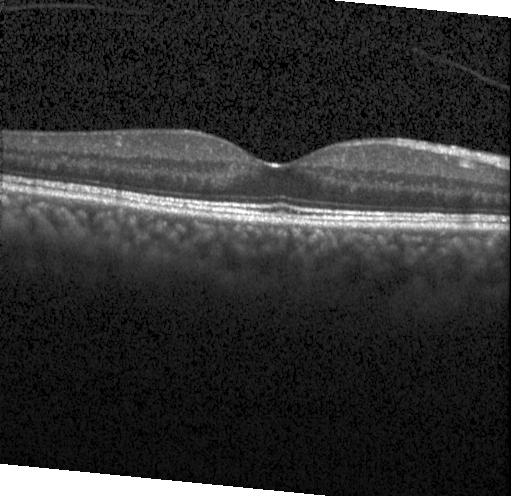 Diagnosis: no CNV, DME, or drusen.